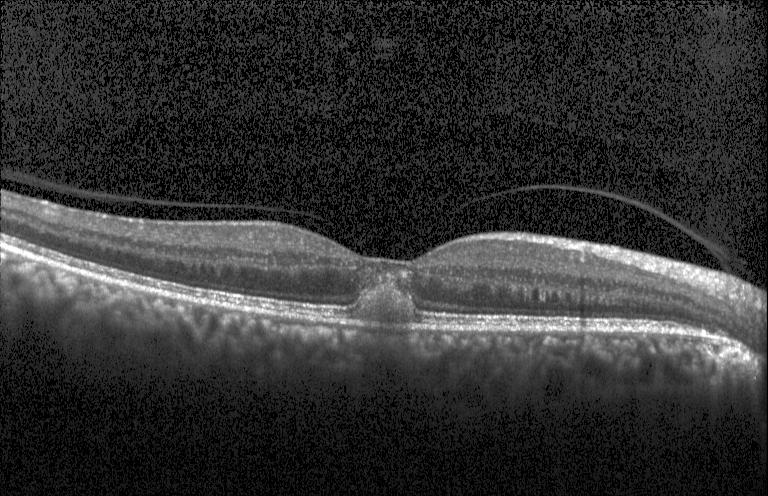 This B-scan demonstrates choroidal neovascularization (CNV).